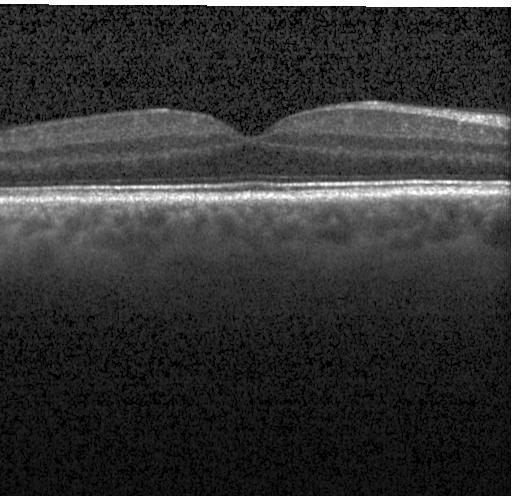 OCT line scan; fovea-centered
This B-scan demonstrates neither choroidal neovascularization, diabetic macular edema, nor drusen.